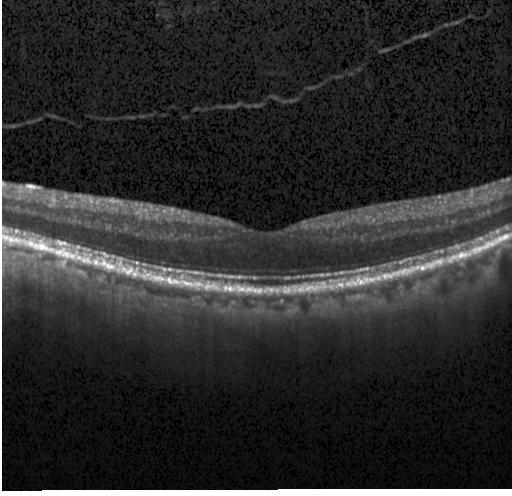

Retinal OCT B-scan
This B-scan demonstrates no CNV, DME, or drusen.